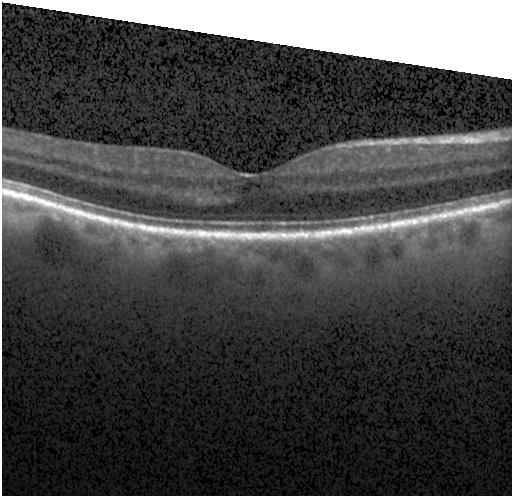 Through the macula, spectral-domain OCT, instrument: Heidelberg Spectralis, retinal OCT B-scan — Finding: no CNV, DME, or drusen.